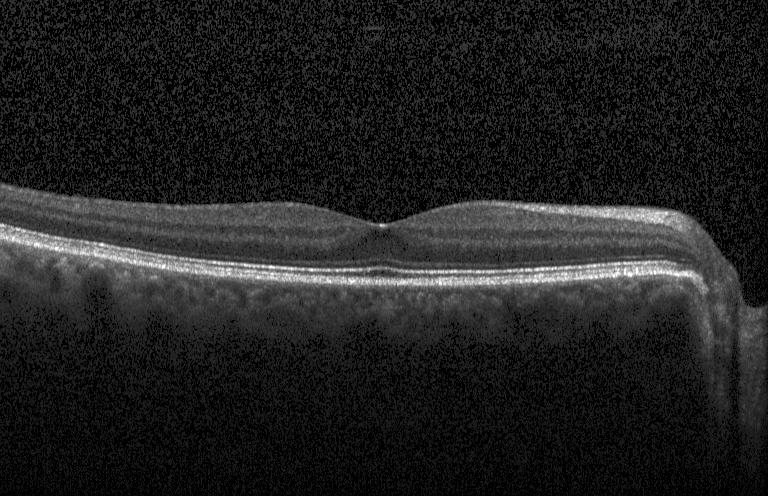
Optical coherence tomography B-scan — Diagnosis: no choroidal neovascularization, diabetic macular edema, or drusen.